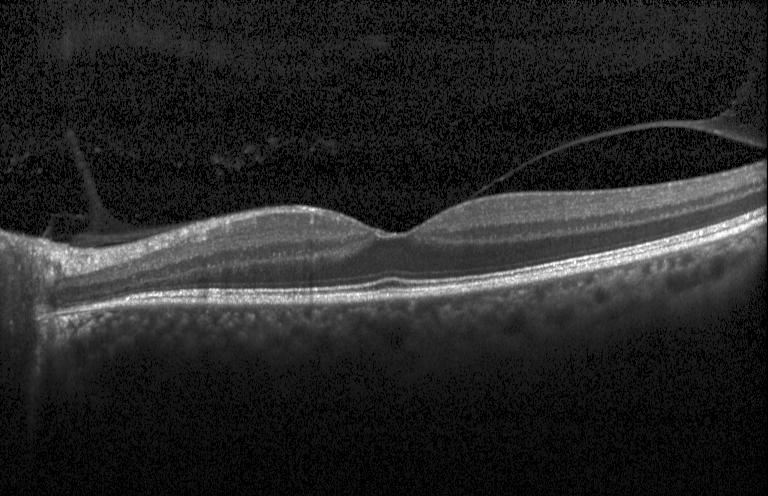 Retinal OCT B-scan · instrument: Heidelberg Spectralis · spectral-domain optical coherence tomography · macular scan — Diagnosis: no choroidal neovascularization, diabetic macular edema, or drusen.